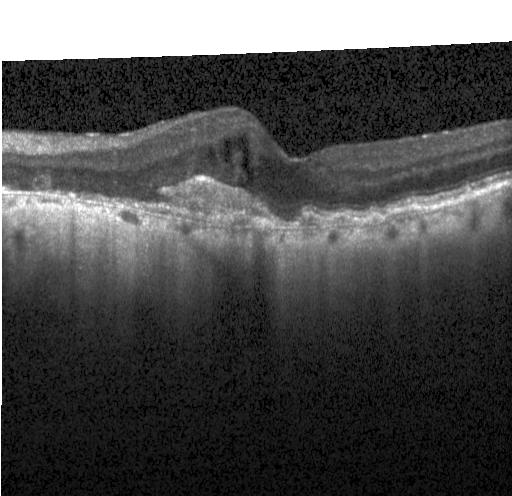 OCT B-scan showing a choroidal neovascular membrane.